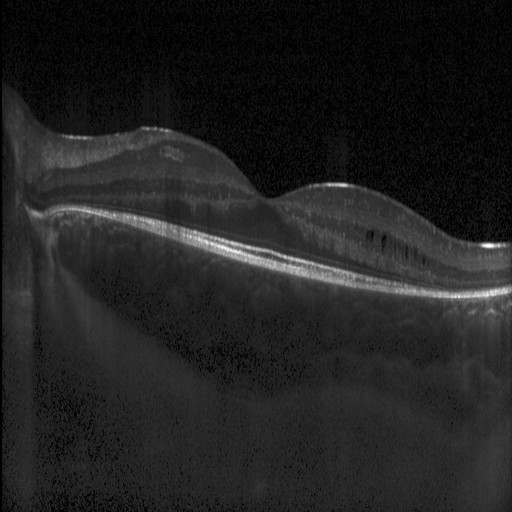
Impression: diabetic macular edema (DME).